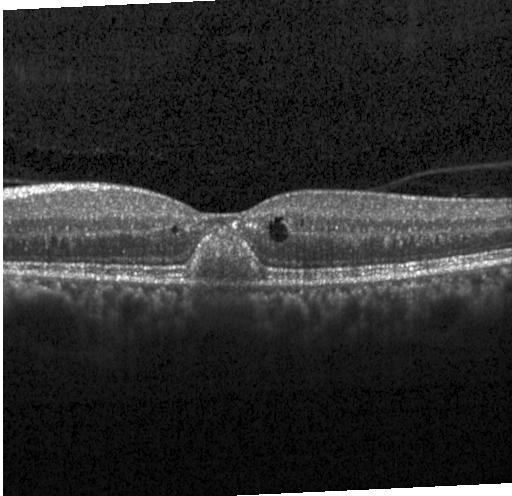
Optical coherence tomography B-scan; through the macula; Heidelberg Spectralis OCT system
The scan shows choroidal neovascularization (CNV).